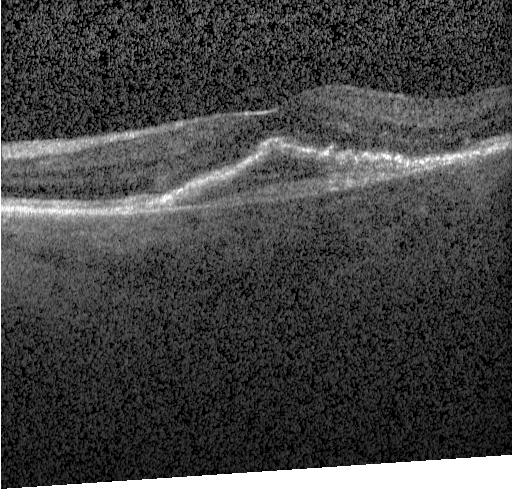 Optical coherence tomography scan, centered on the fovea — OCT finding: CNV.